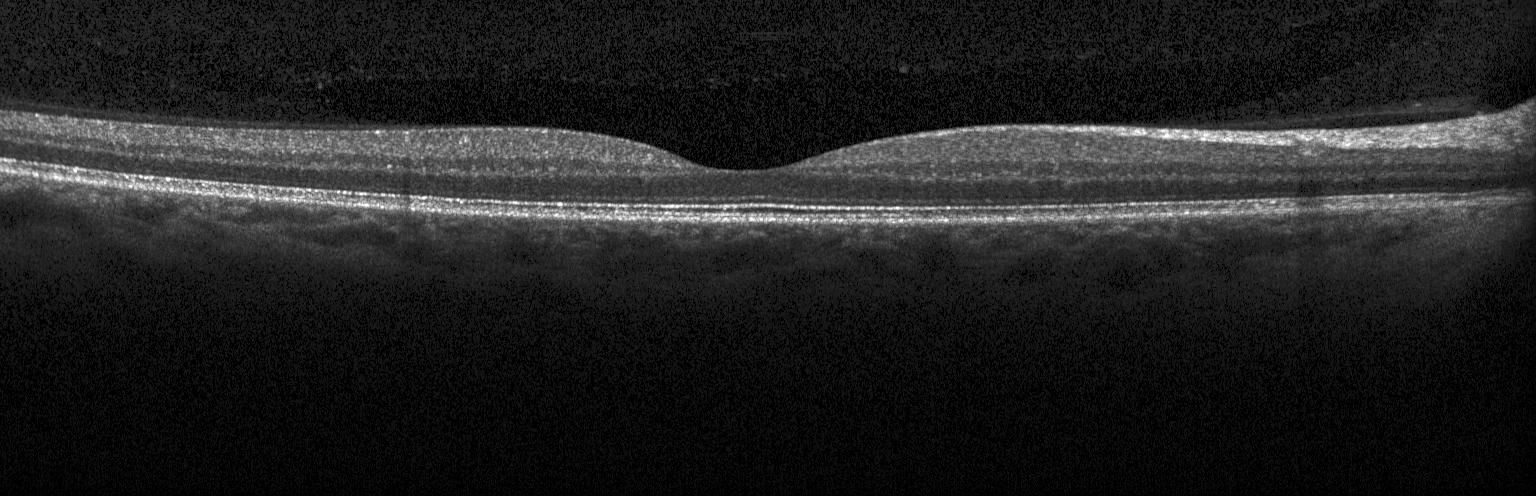 Macular OCT: neither CNV, DME, nor drusen.